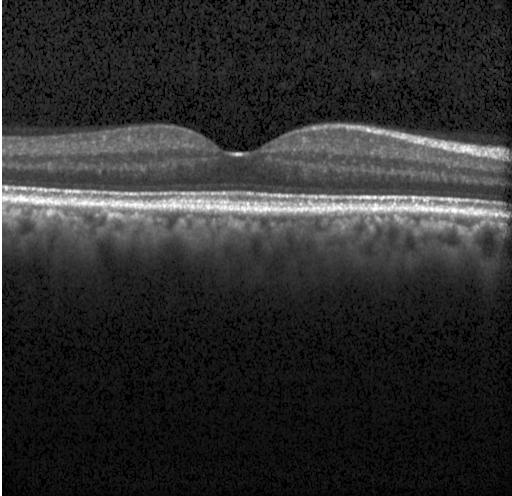
Instrument: Heidelberg Spectralis, spectral-domain optical coherence tomography, OCT B-scan, through the macula. OCT finding: no choroidal neovascularization, no diabetic macular edema, and no drusen.